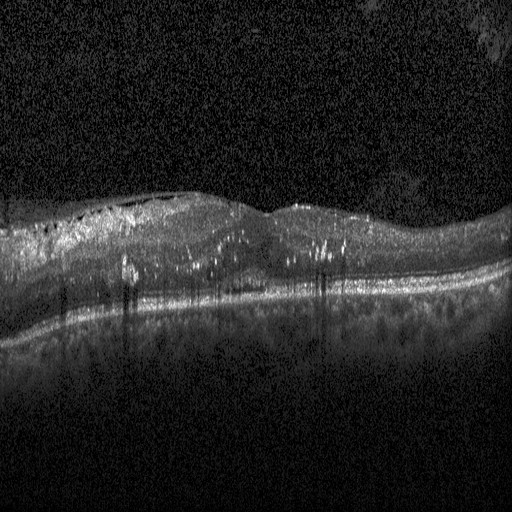 OCT B-scan, Heidelberg Spectralis OCT system, SD-OCT, horizontal scan through the fovea — Finding: diabetic macular edema.